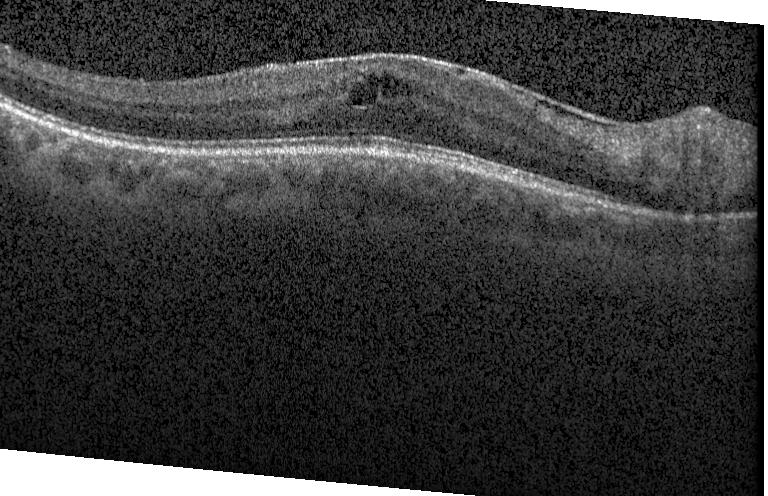

Through the macula · instrument: Heidelberg Spectralis · retinal OCT B-scan — Finding: DME.